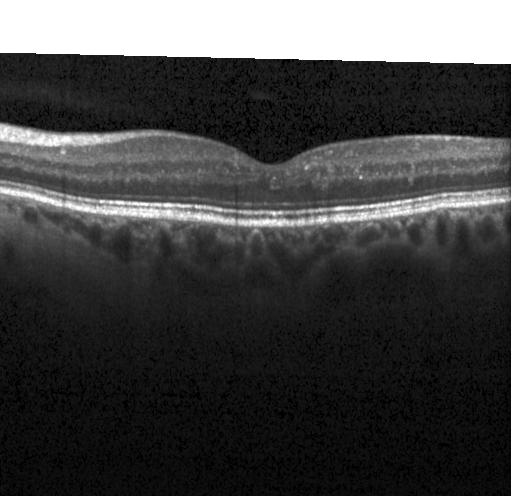

Finding: no CNV, DME, or drusen.